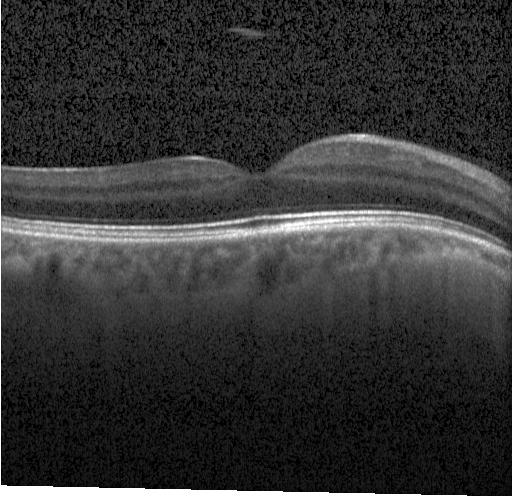

OCT B-scan showing no choroidal neovascularization, diabetic macular edema, or drusen.